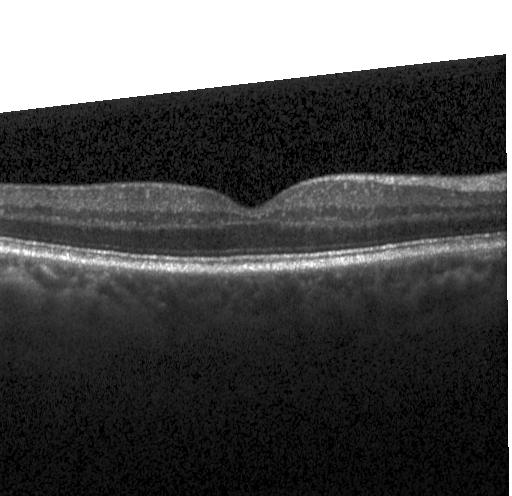
Retinal OCT B-scan, SD-OCT. Finding: no choroidal neovascularization, diabetic macular edema, or drusen.